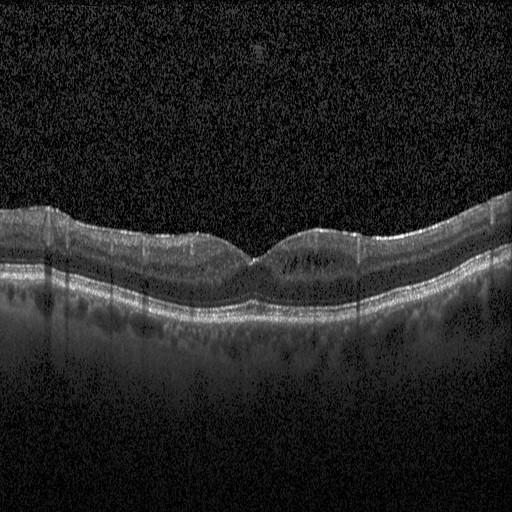 Acquired on a Heidelberg Spectralis; spectral-domain OCT; OCT B-scan.
The scan shows diabetic macular edema (DME).